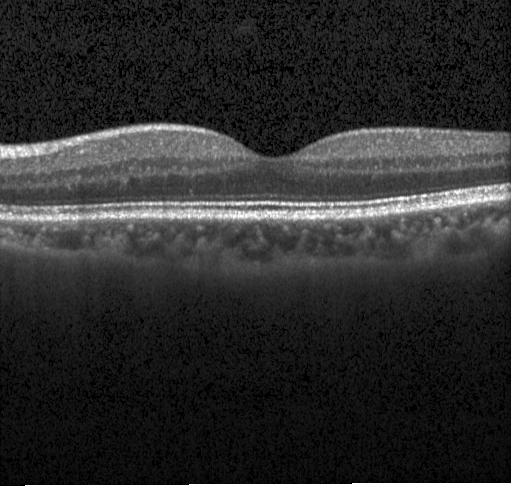
Macular OCT demonstrating no evidence of choroidal neovascularization, diabetic macular edema, or drusen.